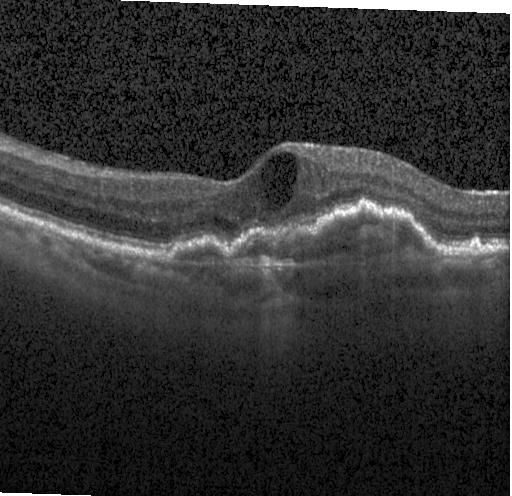 Heidelberg Spectralis; OCT line scan; spectral-domain optical coherence tomography
Assessment: choroidal neovascularization.